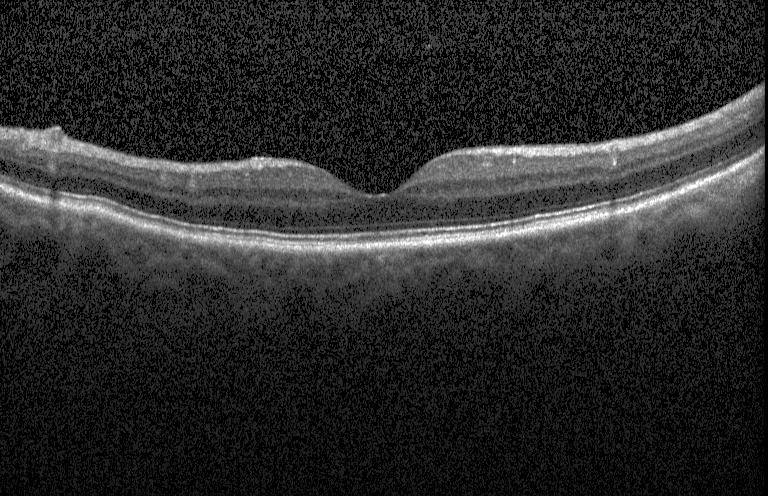
Spectral-domain optical coherence tomography, instrument: Heidelberg Spectralis, macular scan, OCT line scan. The scan shows neither CNV, DME, nor drusen.